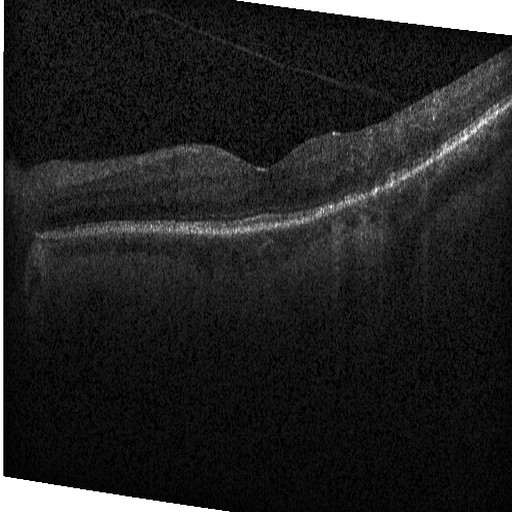 Retinal OCT cross-section. SD-OCT — Finding: diabetic macular edema (DME).